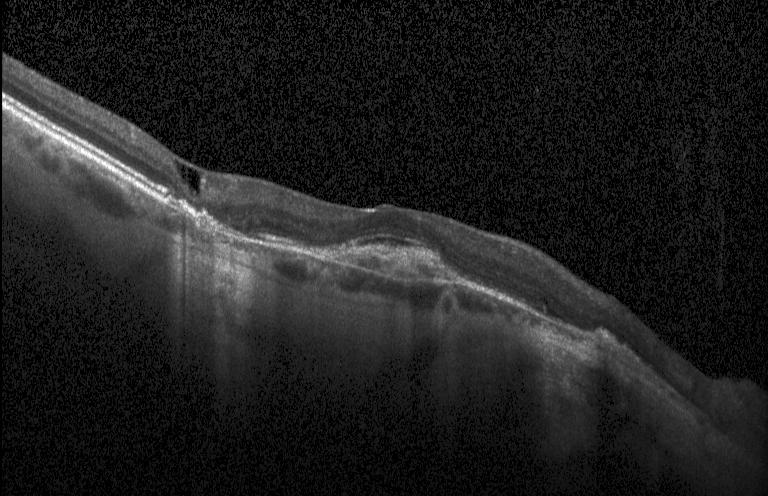
OCT line scan.
Finding: a choroidal neovascular membrane.